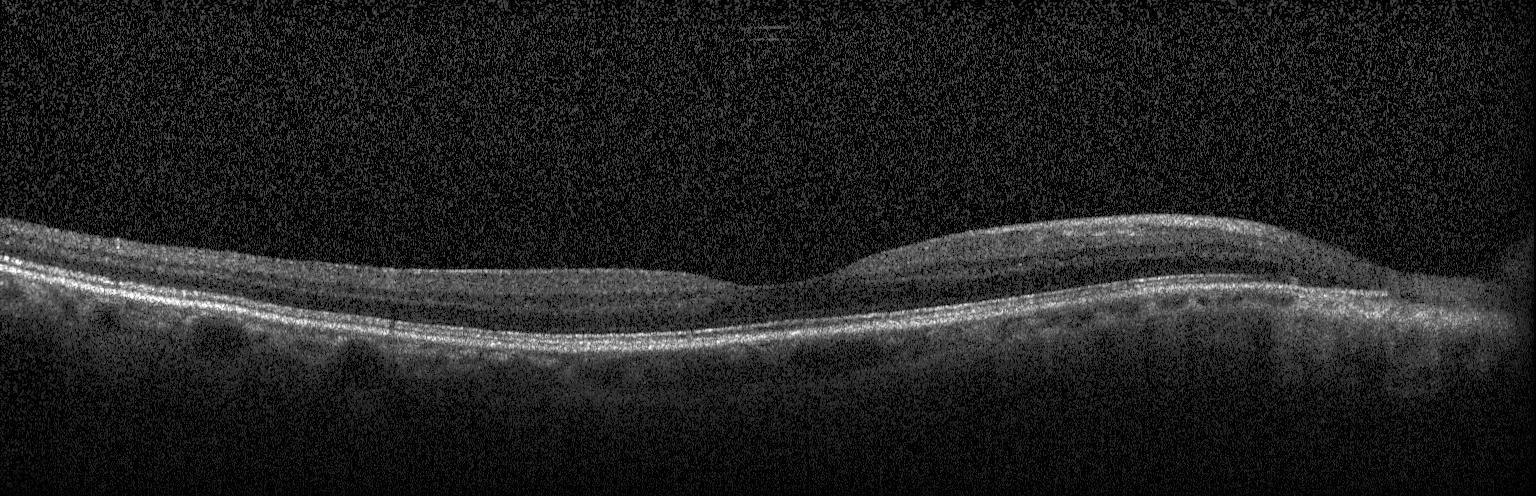
SD-OCT. Optical coherence tomography scan.
Impression: no choroidal neovascularization, diabetic macular edema, or drusen.